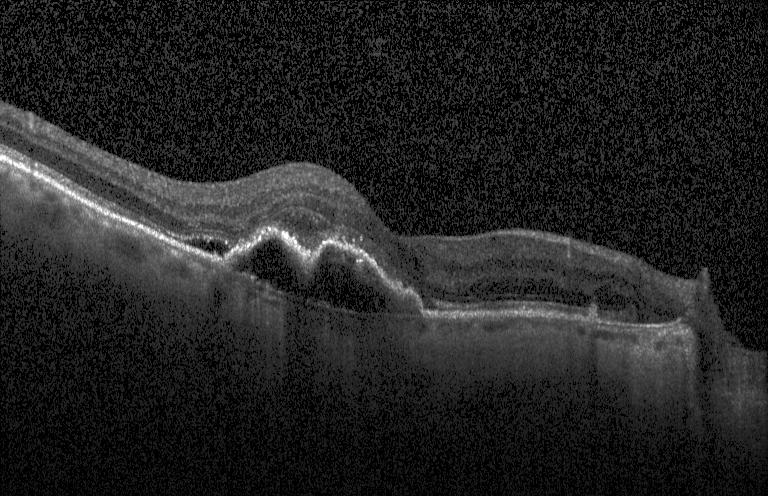 SD-OCT · Heidelberg Spectralis · optical coherence tomography B-scan · centered on the fovea.
Impression: a choroidal neovascular membrane.